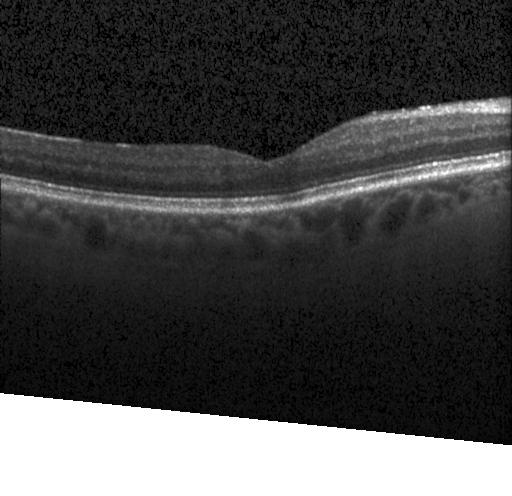 Diagnosis: no evidence of CNV, DME, or drusen.